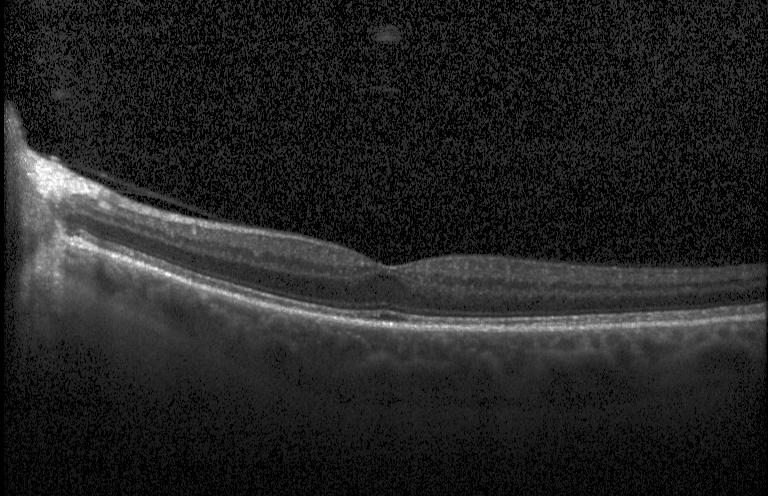

Heidelberg Spectralis, through the macula, OCT B-scan. Diagnosis: no evidence of CNV, DME, or drusen.